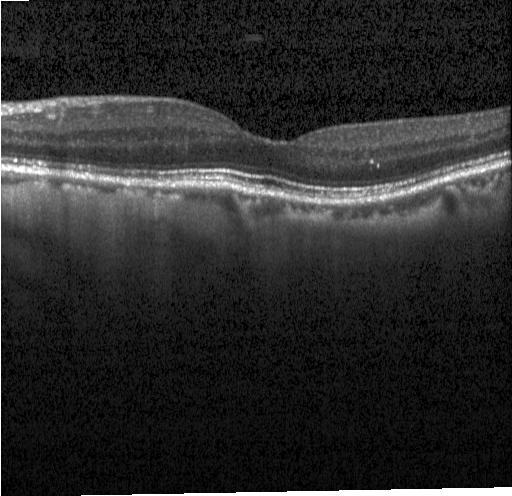
Spectral-domain OCT B-scan: neither choroidal neovascularization, diabetic macular edema, nor drusen.